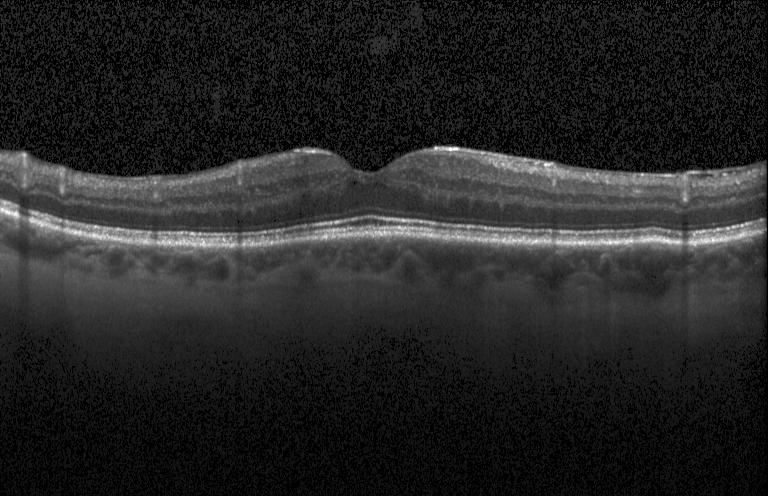

Spectral-domain optical coherence tomography; acquired on a Heidelberg Spectralis; OCT B-scan; fovea-centered — No choroidal neovascularization, diabetic macular edema, or drusen.